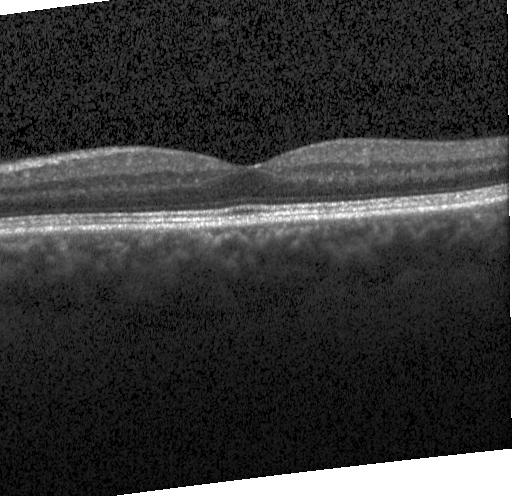

OCT B-scan, SD-OCT. The scan shows no evidence of CNV, DME, or drusen.